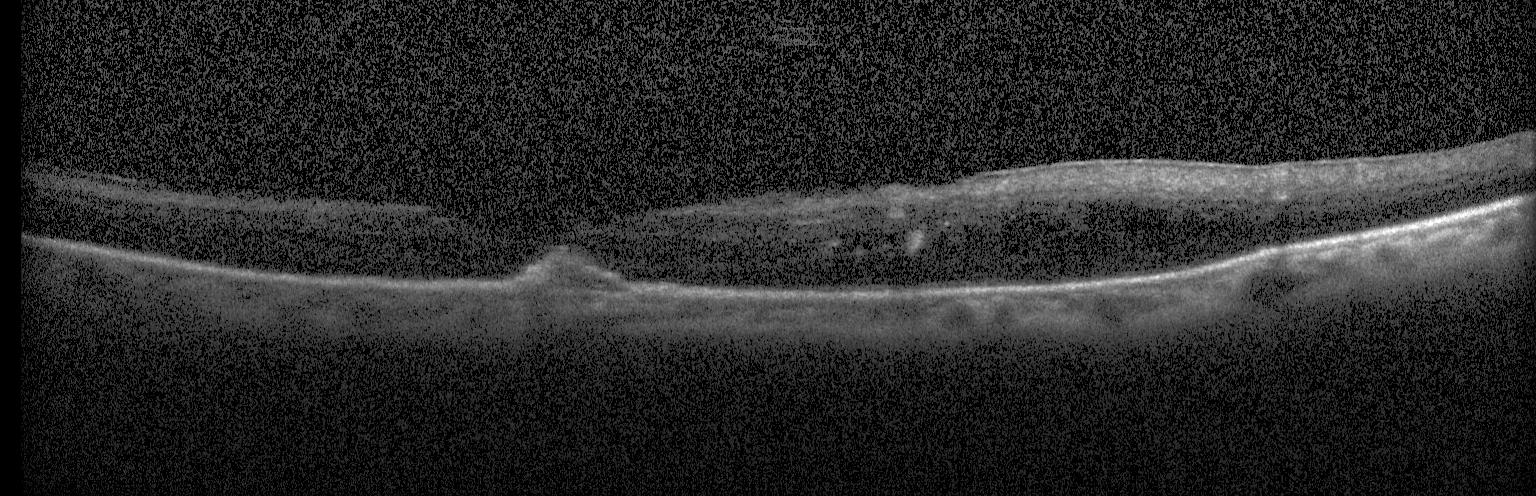
OCT B-scan.
This B-scan demonstrates a choroidal neovascular membrane.